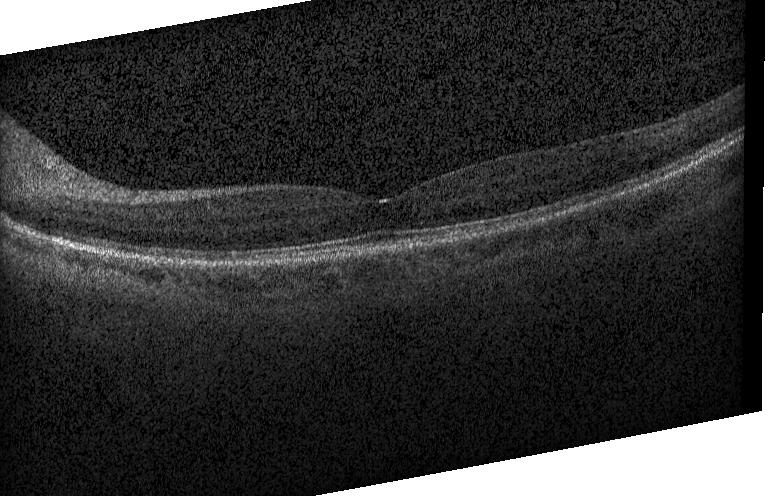
Spectral-domain OCT, Heidelberg Spectralis OCT system, retinal OCT cross-section, through the macula — Finding: no choroidal neovascularization, no diabetic macular edema, and no drusen.